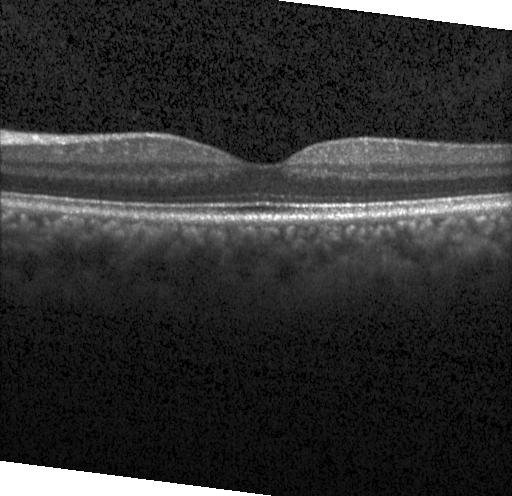

Retinal OCT cross-section. Horizontal scan through the fovea. Diagnosis: no choroidal neovascularization, no diabetic macular edema, and no drusen.